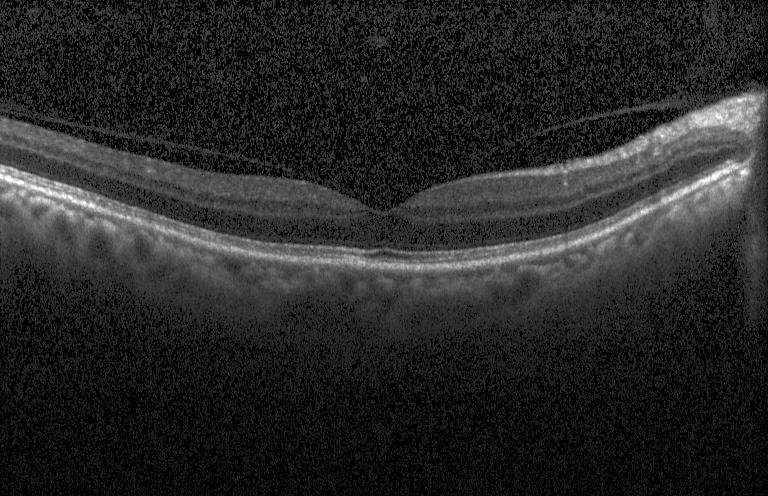

OCT line scan; horizontal scan through the fovea
Diagnosis: no choroidal neovascularization, no diabetic macular edema, and no drusen.